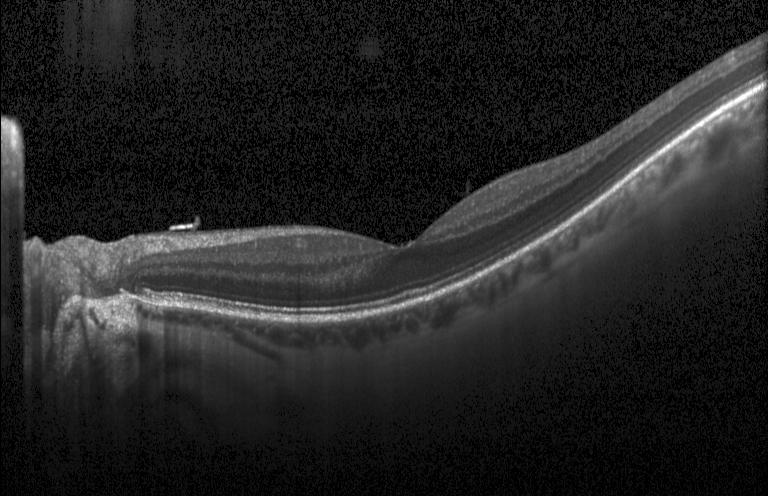
Spectral-domain OCT. Optical coherence tomography scan. Finding: no evidence of CNV, DME, or drusen.